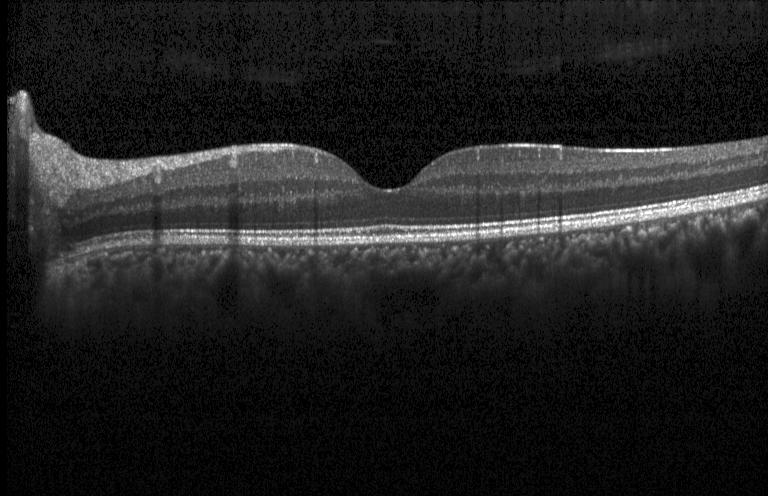 Retinal OCT cross-section, macular scan, instrument: Heidelberg Spectralis, spectral-domain optical coherence tomography. Macular OCT: no CNV, DME, or drusen.